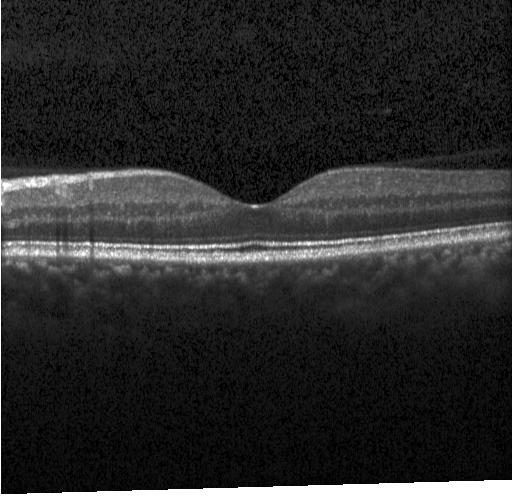

Assessment: neither choroidal neovascularization, diabetic macular edema, nor drusen.